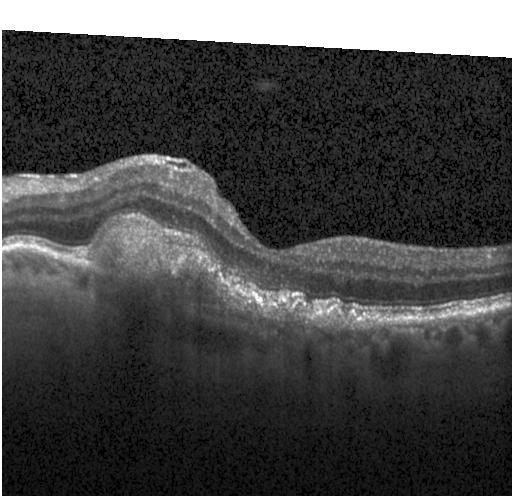 Diagnosis: choroidal neovascularization.